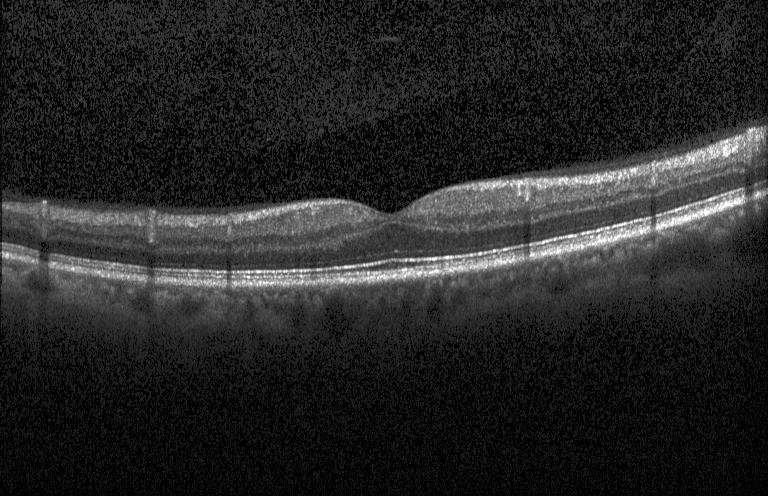 Optical coherence tomography scan.
Dx: neither CNV, DME, nor drusen.